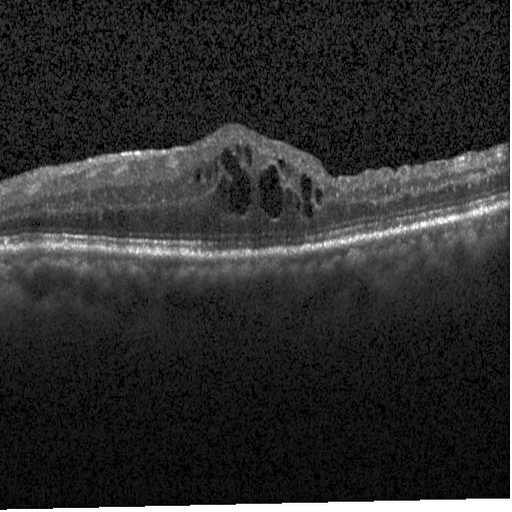
OCT finding: diabetic macular edema (DME).